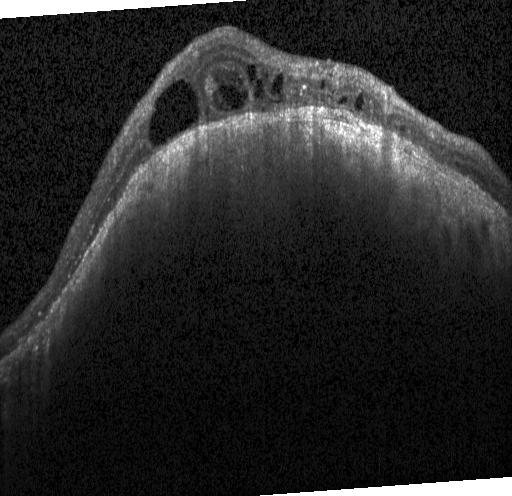

Centered on the fovea, retinal OCT B-scan, spectral-domain OCT, instrument: Heidelberg Spectralis — Dx: diabetic macular edema.